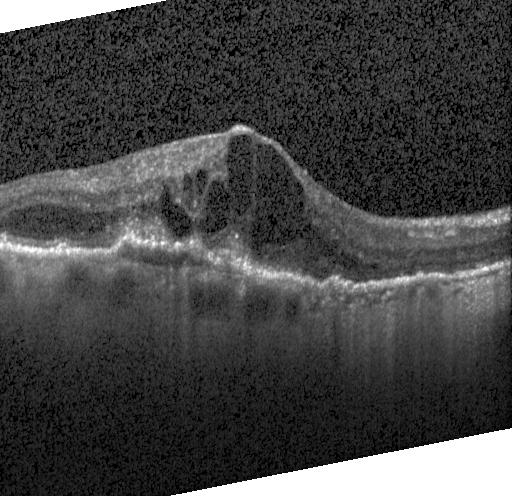
Instrument: Heidelberg Spectralis · OCT B-scan
Impression: a choroidal neovascular membrane.